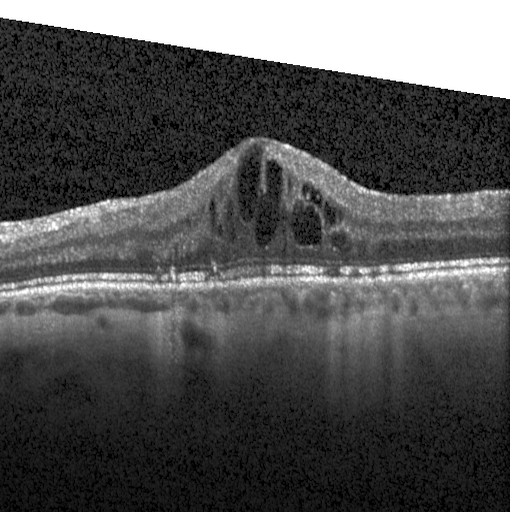

Impression: DME.